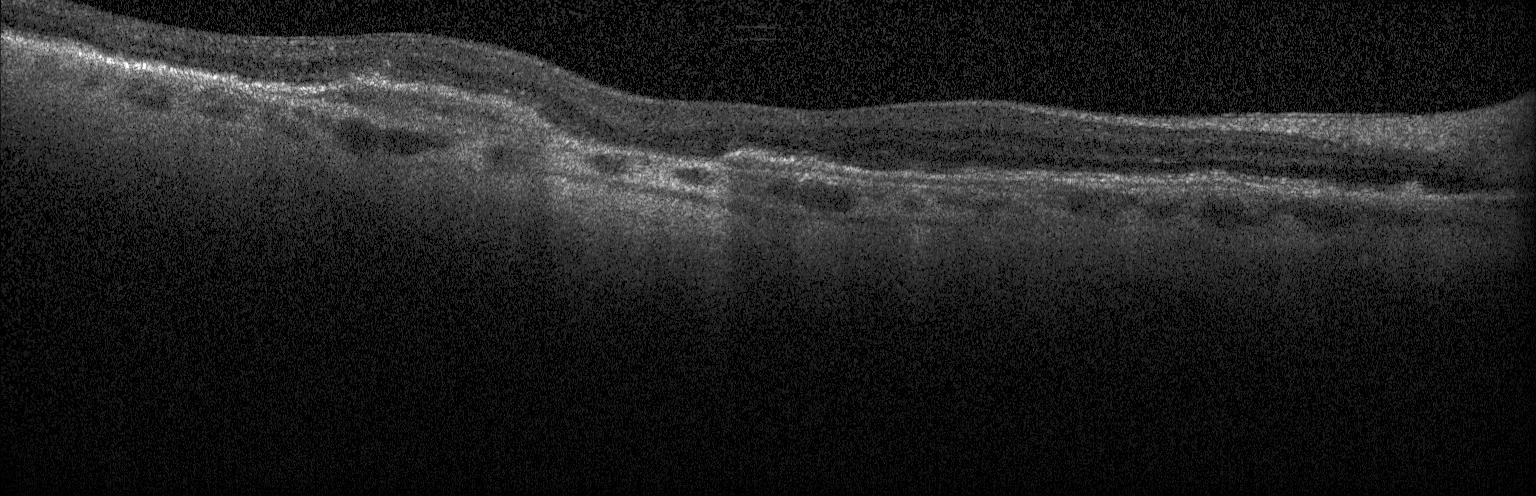 Optical coherence tomography scan; centered on the fovea; Heidelberg Spectralis OCT system; spectral-domain optical coherence tomography
Impression: a choroidal neovascular membrane.